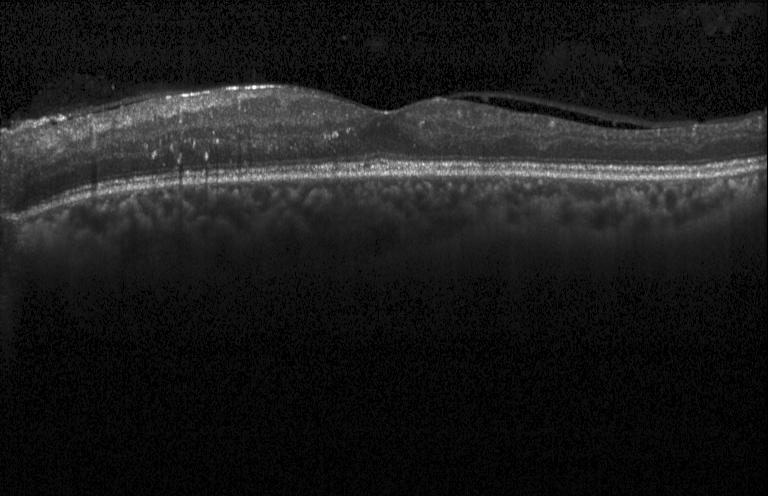
Instrument: Heidelberg Spectralis. Optical coherence tomography B-scan. Centered on the fovea. The scan shows diabetic macular edema (DME).